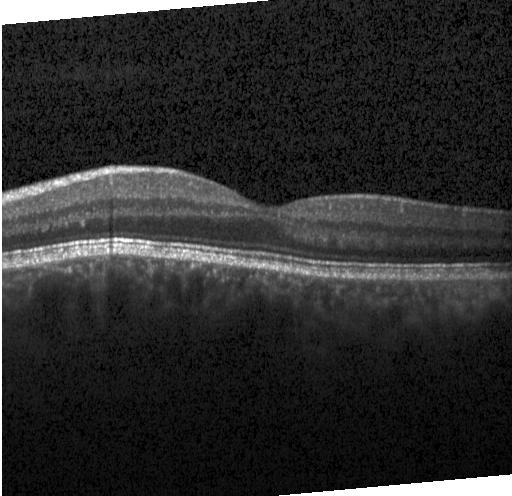
OCT B-scan
Diagnosis: no choroidal neovascularization, diabetic macular edema, or drusen.